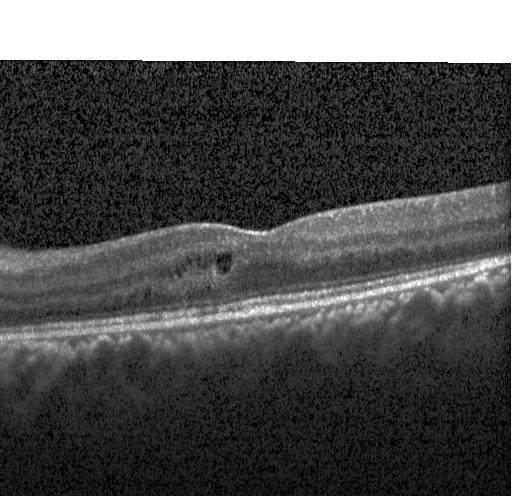

Centered on the fovea; OCT line scan; spectral-domain optical coherence tomography
Diagnosis: DME.